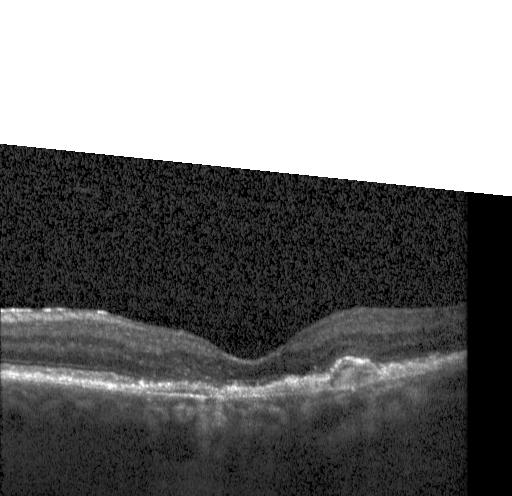

OCT B-scan.
Dx: choroidal neovascularization (CNV).